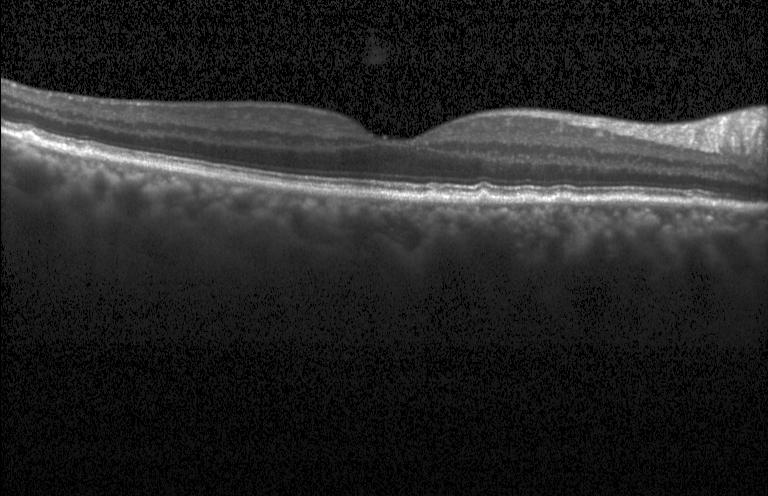
Optical coherence tomography scan. Drusen.